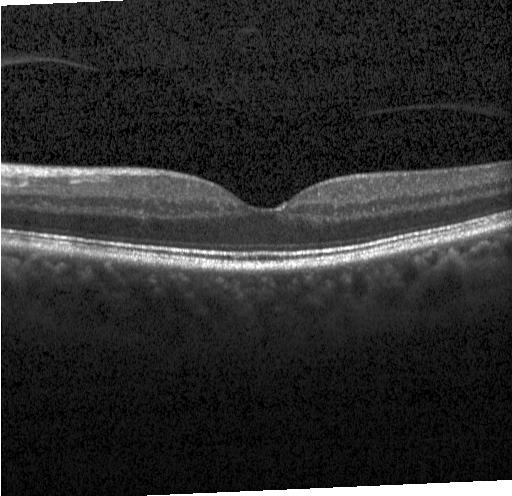
Acquired on a Heidelberg Spectralis. Spectral-domain OCT. Fovea-centered. Optical coherence tomography B-scan
Diagnosis: neither choroidal neovascularization, diabetic macular edema, nor drusen.